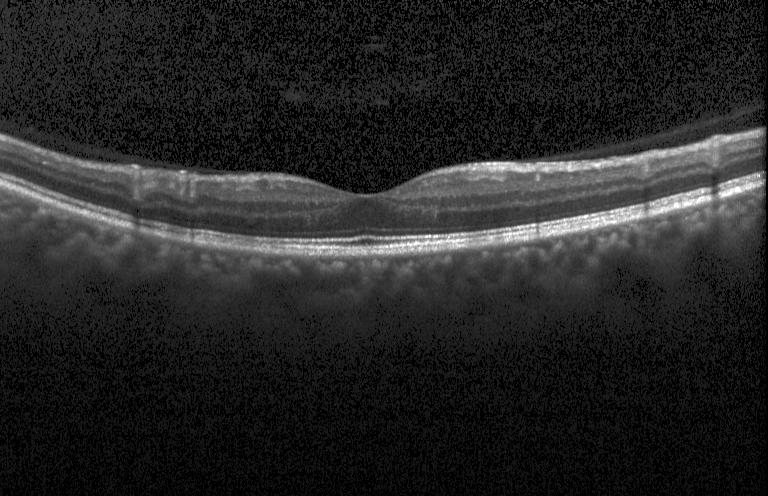 Retinal OCT B-scan. Acquired on a Heidelberg Spectralis. SD-OCT.
Finding: no choroidal neovascularization, no diabetic macular edema, and no drusen.